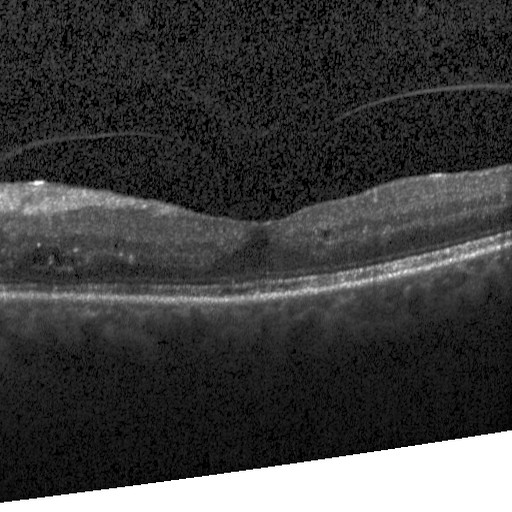 Impression: DME.